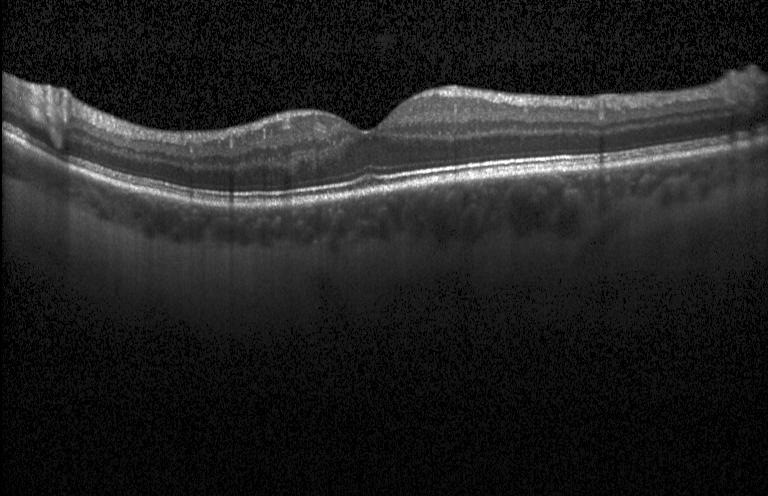

Impression: no evidence of CNV, DME, or drusen.